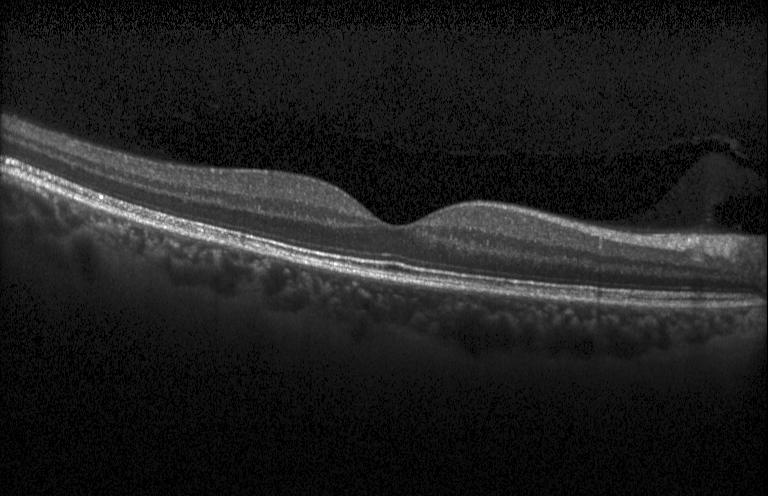 OCT line scan. Acquired on a Heidelberg Spectralis. Fovea-centered — Dx: no evidence of CNV, DME, or drusen.